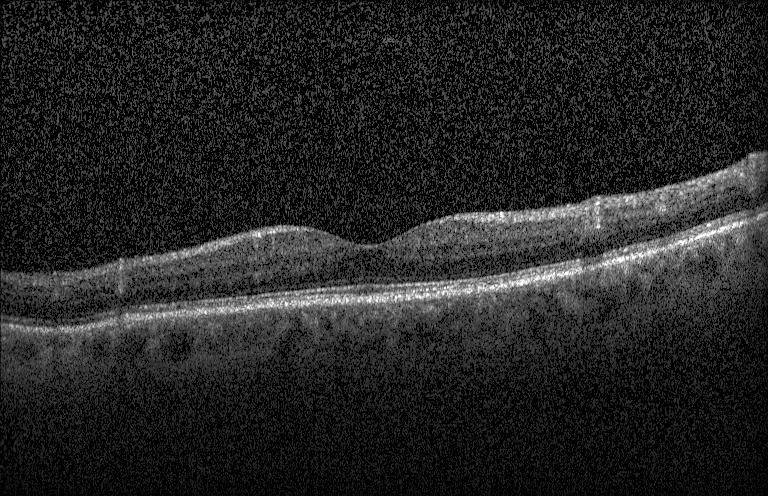 Optical coherence tomography B-scan. Assessment: no evidence of choroidal neovascularization, diabetic macular edema, or drusen.